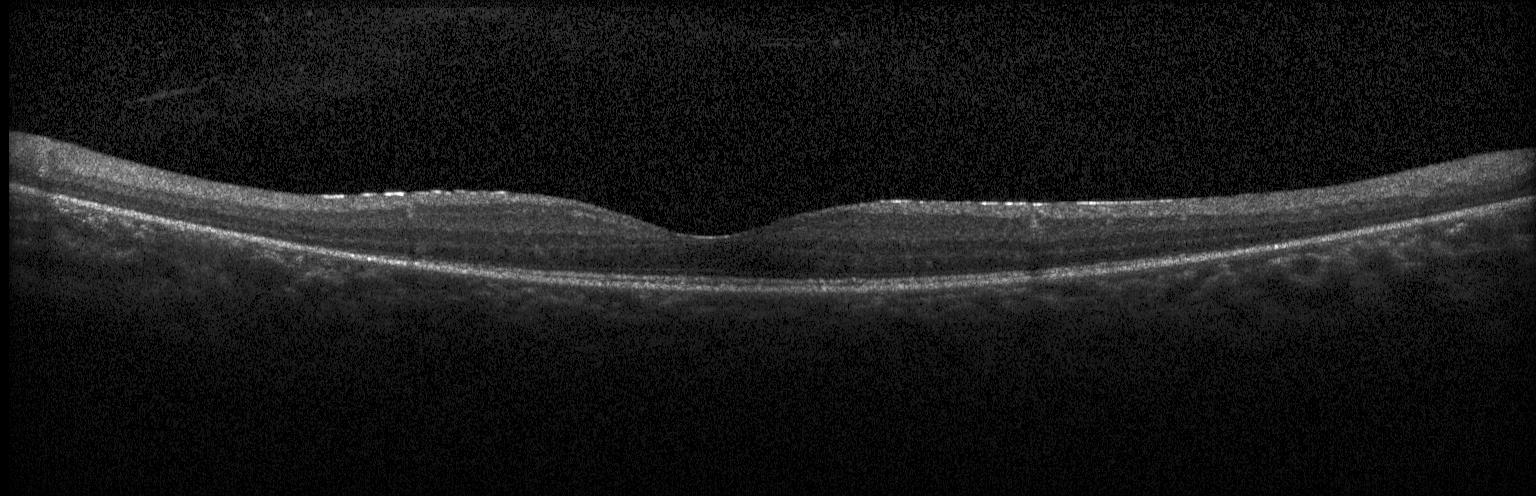 Assessment: neither choroidal neovascularization, diabetic macular edema, nor drusen.